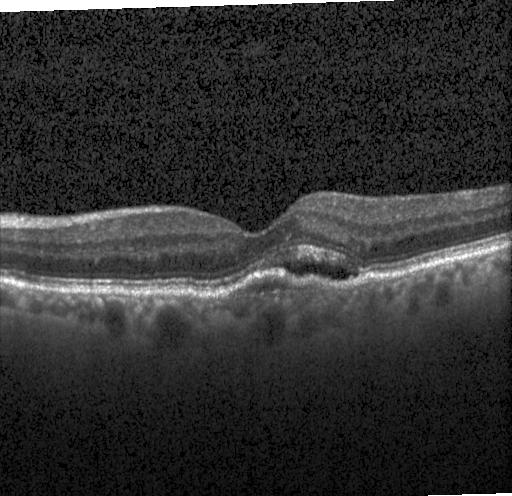

Optical coherence tomography scan, acquired on a Heidelberg Spectralis
Impression: a choroidal neovascular membrane.